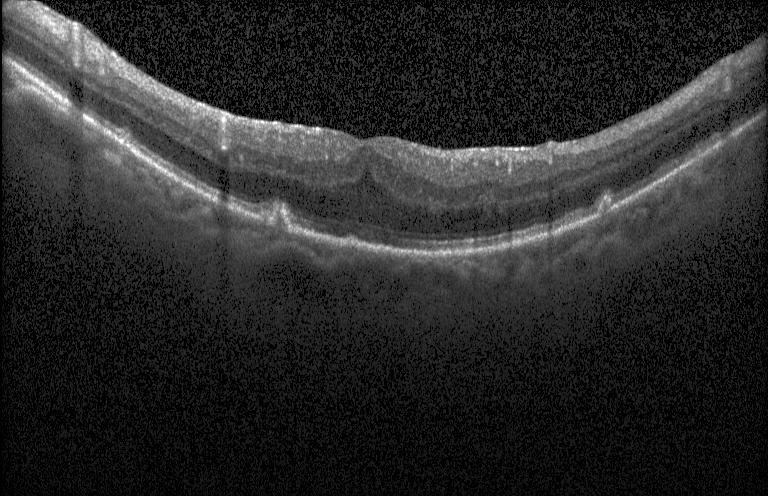 Heidelberg Spectralis OCT system. Fovea-centered. Spectral-domain optical coherence tomography. Retinal OCT cross-section — Dx: sub-RPE drusenoid deposits.